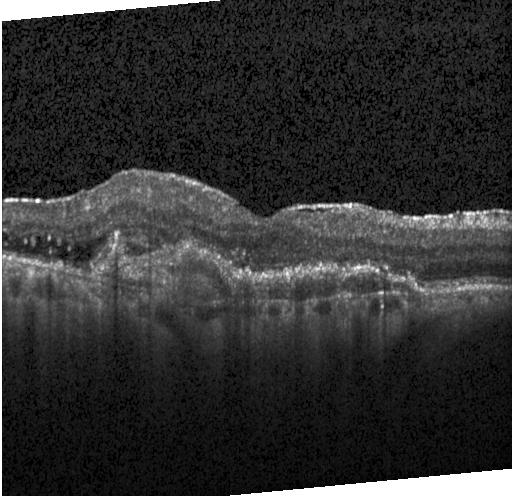

Finding: choroidal neovascularization (CNV).